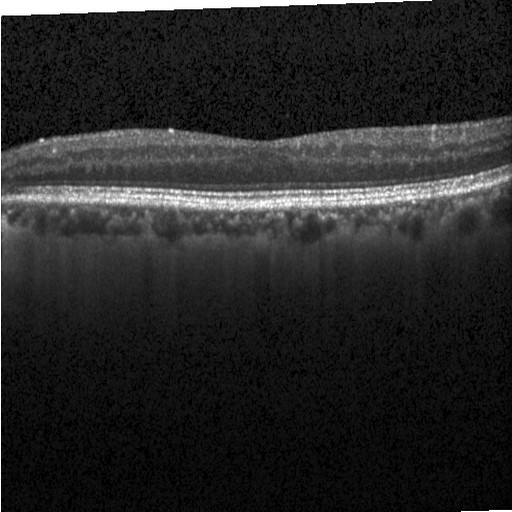
Impression: diabetic macular edema.